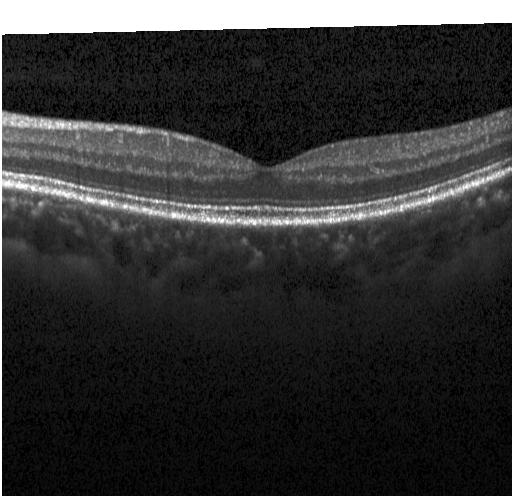

Diagnosis: neither CNV, DME, nor drusen.